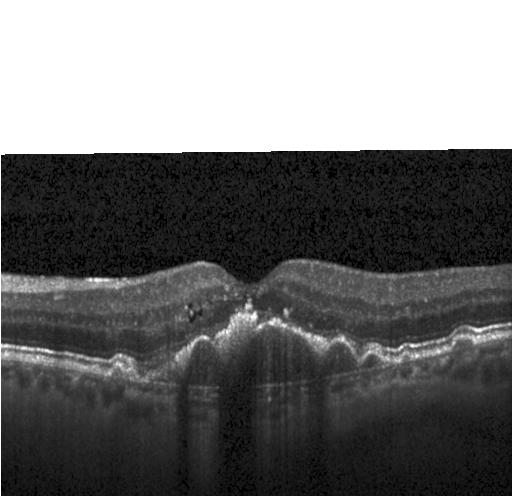
The scan shows a choroidal neovascular membrane.